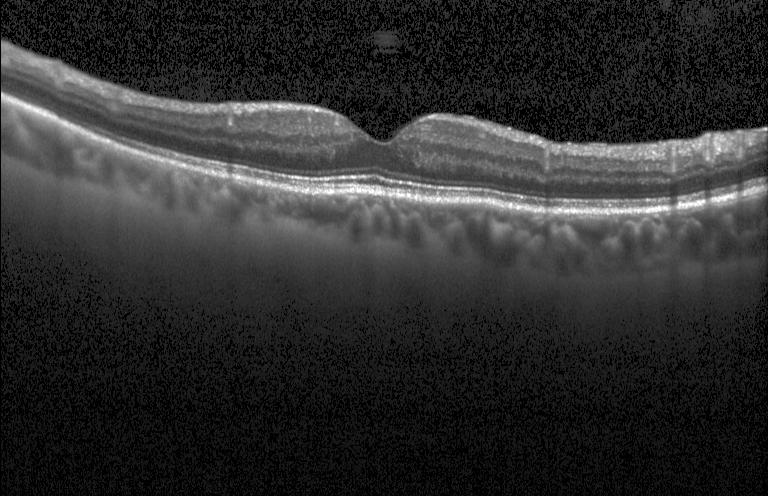 Optical coherence tomography scan. This B-scan demonstrates no choroidal neovascularization, diabetic macular edema, or drusen.